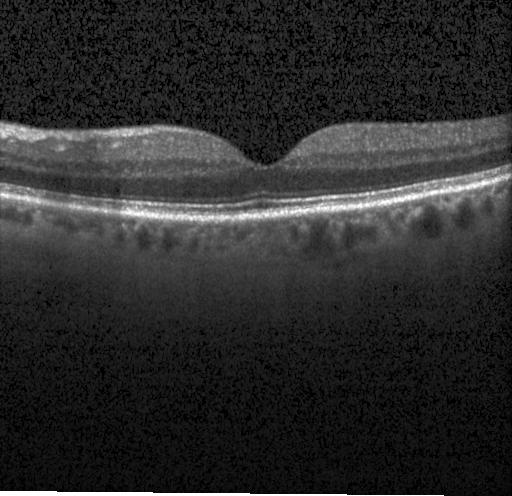 Optical coherence tomography scan — The scan shows no choroidal neovascularization, diabetic macular edema, or drusen.